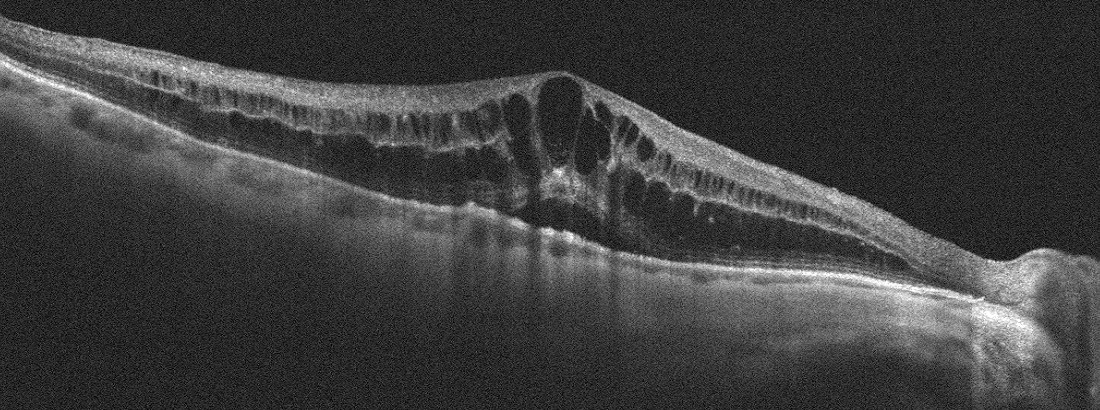

Optical coherence tomography B-scan · fovea-centered · Optovue Avanti RTVue XR.
Macular OCT: RVO.